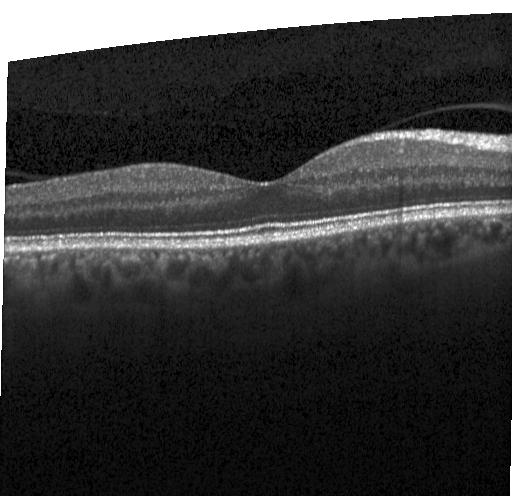

Retinal OCT cross-section.
This B-scan demonstrates no choroidal neovascularization, no diabetic macular edema, and no drusen.